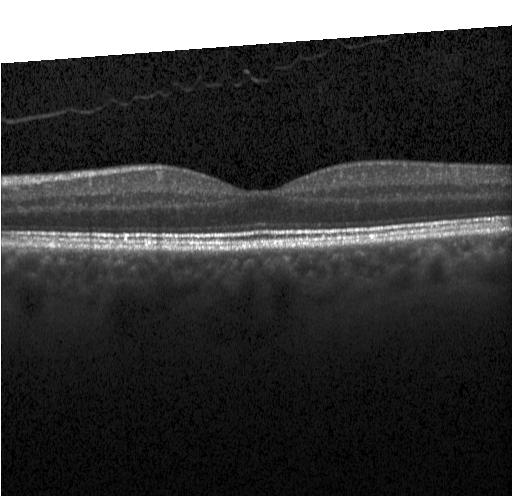

Spectral-domain optical coherence tomography · OCT line scan
Impression: no evidence of choroidal neovascularization, diabetic macular edema, or drusen.